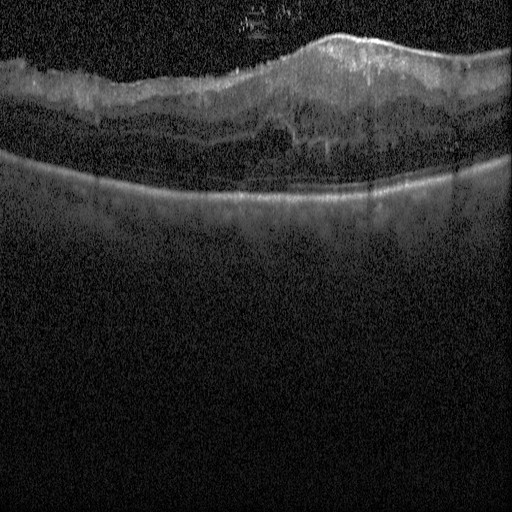 Spectral-domain OCT B-scan: diabetic macular edema.